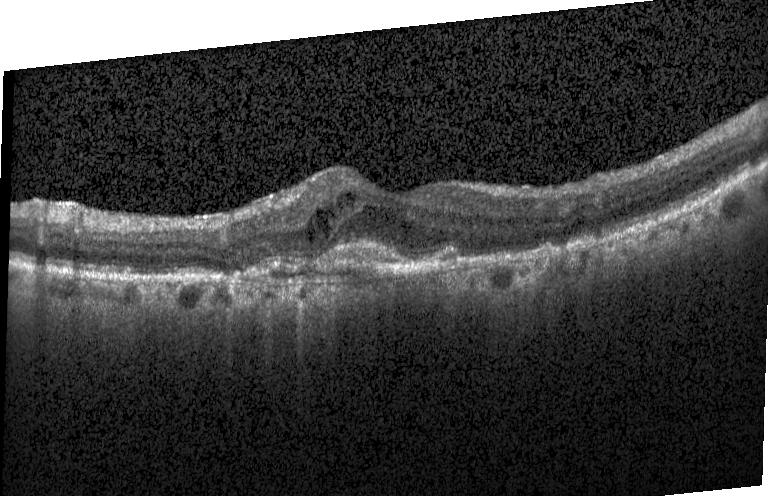

OCT B-scan showing choroidal neovascularization (CNV).